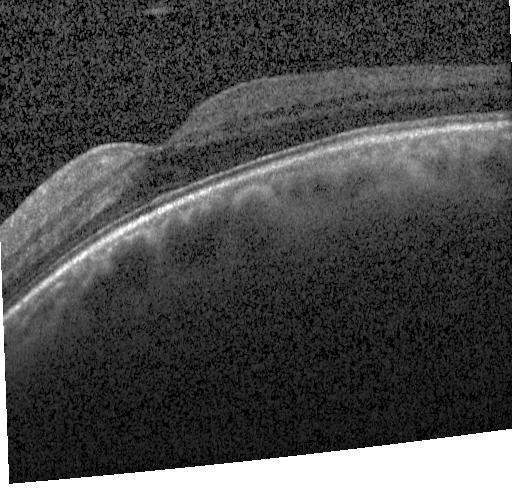 Instrument: Heidelberg Spectralis; retinal OCT cross-section
Diagnosis: neither CNV, DME, nor drusen.